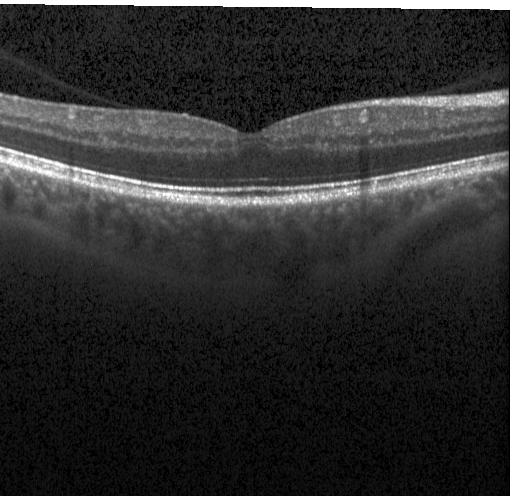
SD-OCT; OCT line scan — The scan shows neither choroidal neovascularization, diabetic macular edema, nor drusen.